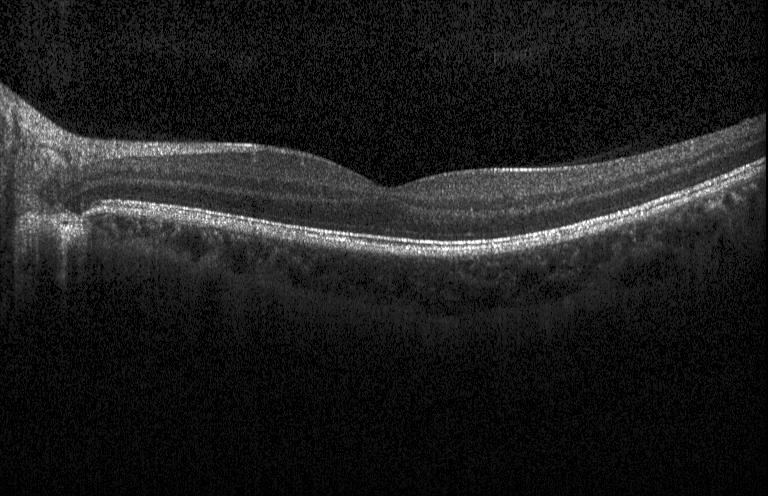
Through the macula; optical coherence tomography B-scan
No CNV, no DME, and no drusen.